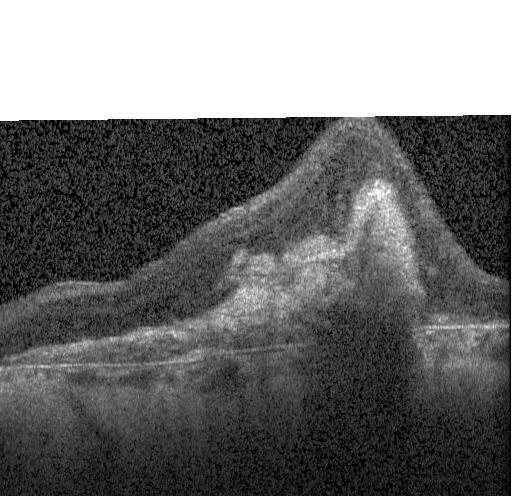

Macular scan, SD-OCT, OCT line scan.
OCT finding: CNV.